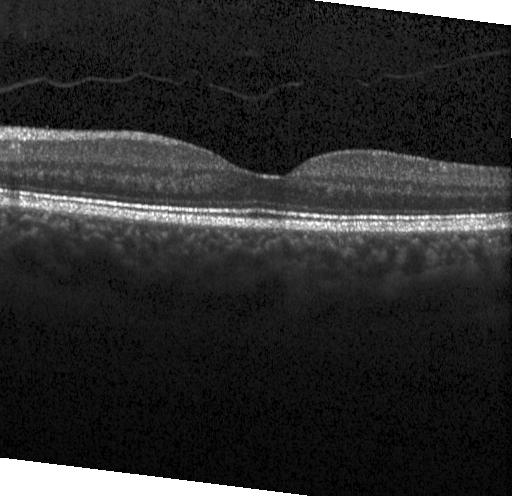

Finding: no choroidal neovascularization, no diabetic macular edema, and no drusen.